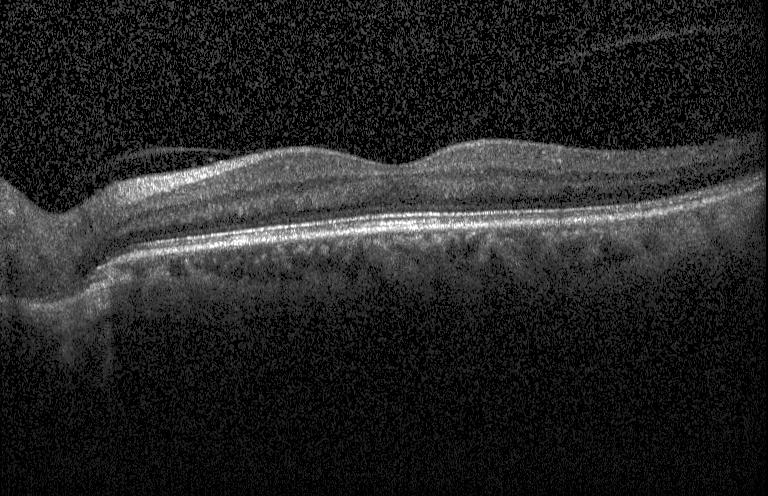

Optical coherence tomography B-scan. SD-OCT. Acquired on a Heidelberg Spectralis. Macular scan. No CNV, no DME, and no drusen.